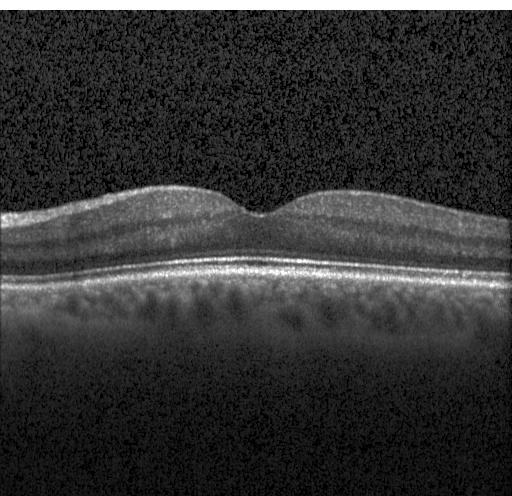 This B-scan demonstrates no choroidal neovascularization, diabetic macular edema, or drusen.